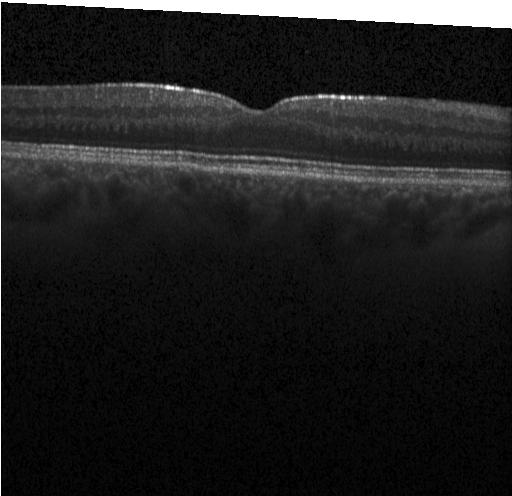

OCT B-scan showing no CNV, no DME, and no drusen.